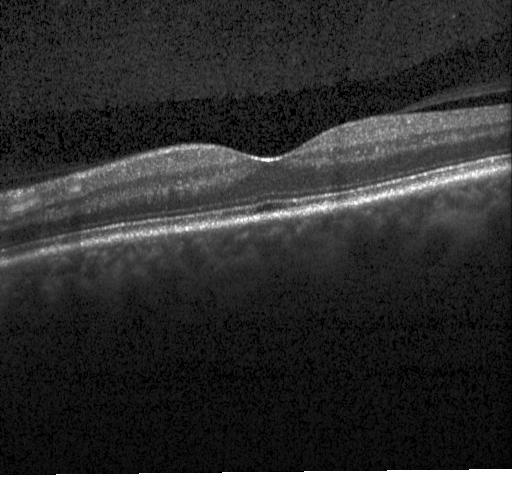

Through the macula. OCT B-scan. Heidelberg Spectralis OCT system. Spectral-domain optical coherence tomography.
Impression: no evidence of CNV, DME, or drusen.